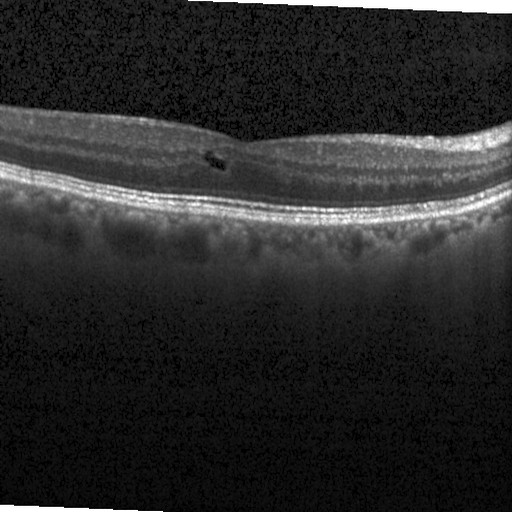

Diagnosis: diabetic macular edema.